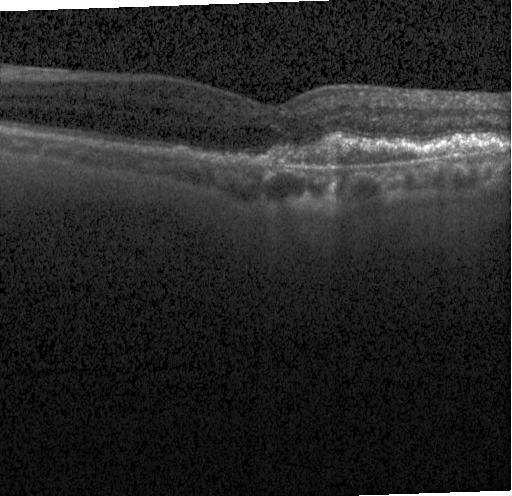
Instrument: Heidelberg Spectralis; optical coherence tomography scan
Impression: a choroidal neovascular membrane.